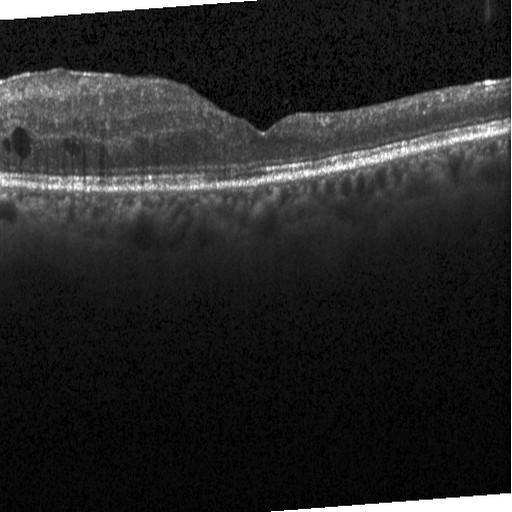

OCT line scan. Instrument: Heidelberg Spectralis. Centered on the fovea
Impression: diabetic macular edema.